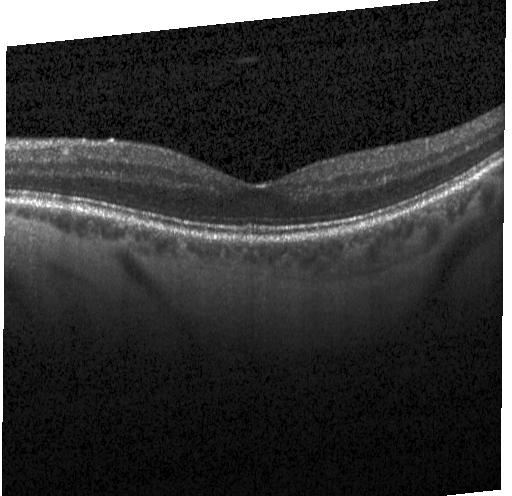
Spectral-domain OCT; instrument: Heidelberg Spectralis; fovea-centered; OCT B-scan
Dx: no evidence of CNV, DME, or drusen.